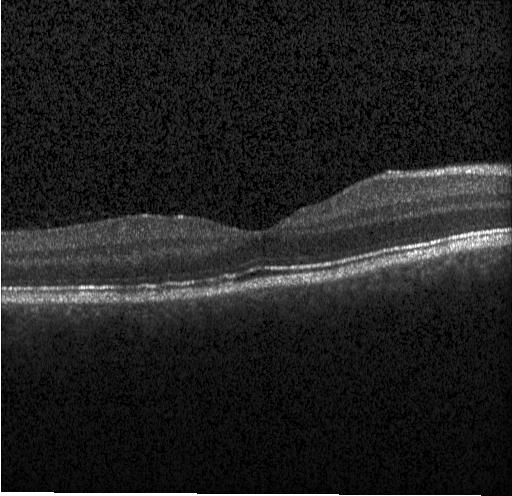 Spectral-domain OCT; horizontal scan through the fovea; retinal OCT B-scan; instrument: Heidelberg Spectralis — Diagnosis: neither CNV, DME, nor drusen.